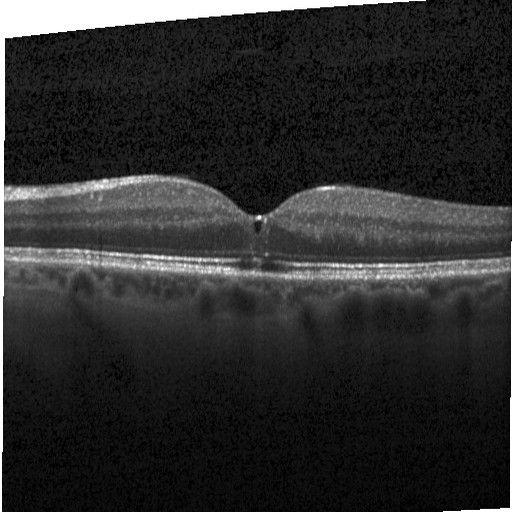

Retinal OCT B-scan, horizontal scan through the fovea, Heidelberg Spectralis OCT system. Impression: DME.